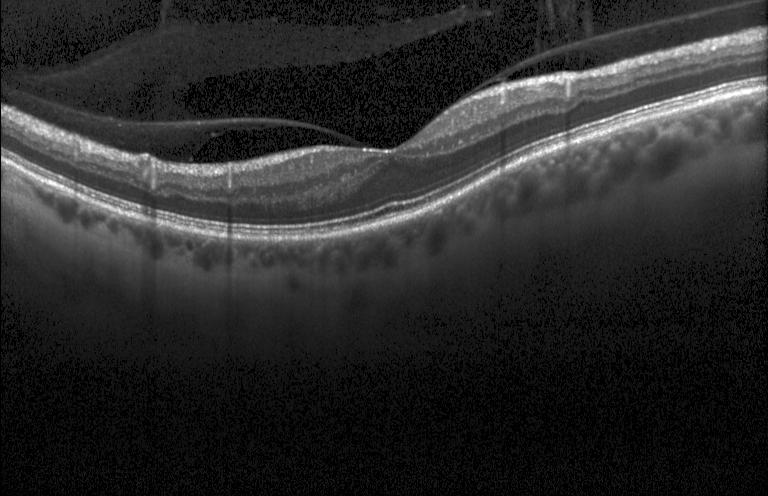

Spectral-domain optical coherence tomography. OCT B-scan. Acquired on a Heidelberg Spectralis. Macular OCT: no evidence of choroidal neovascularization, diabetic macular edema, or drusen.